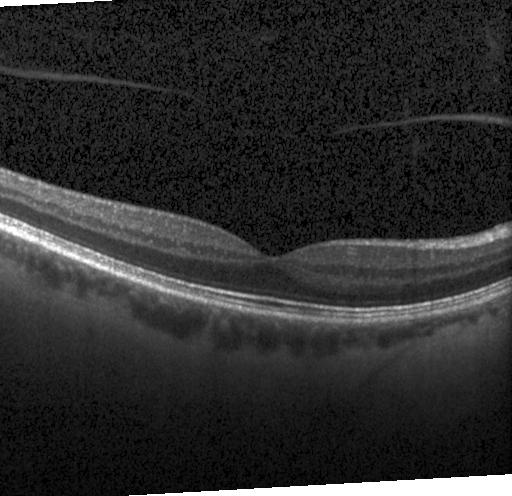

Heidelberg Spectralis · macular scan · SD-OCT · OCT B-scan
Impression: no CNV, no DME, and no drusen.